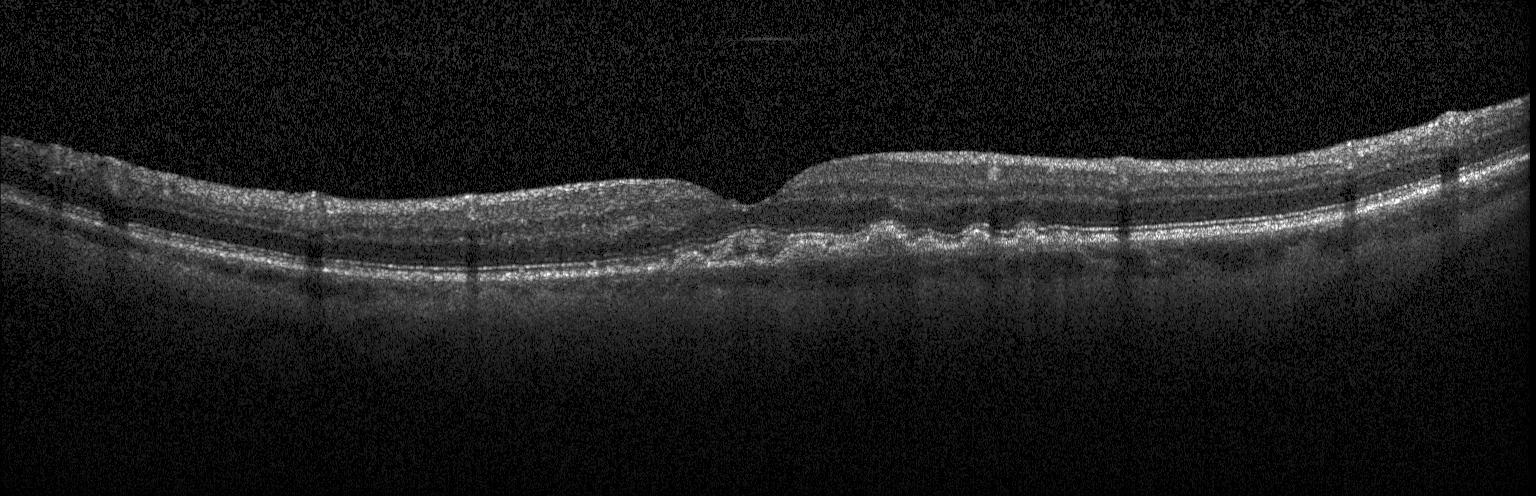 Retinal OCT B-scan — Macular OCT: drusen.